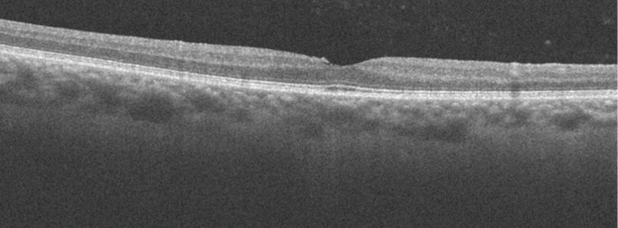 OCT line scan — Assessment: AMD.